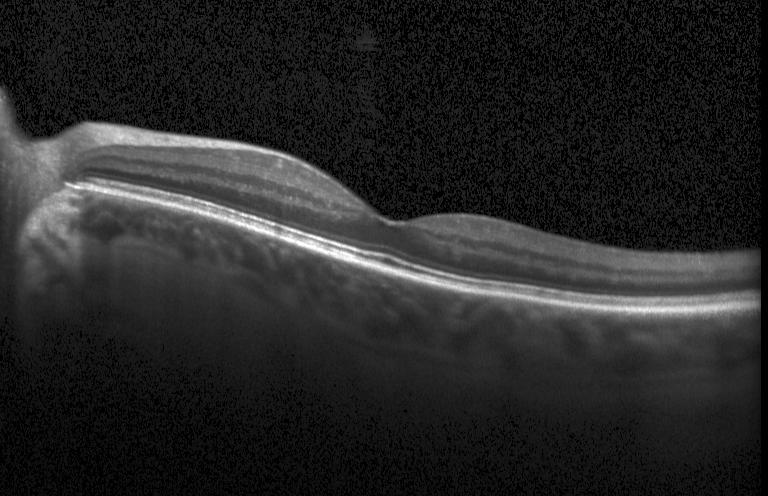
Dx: neither choroidal neovascularization, diabetic macular edema, nor drusen.